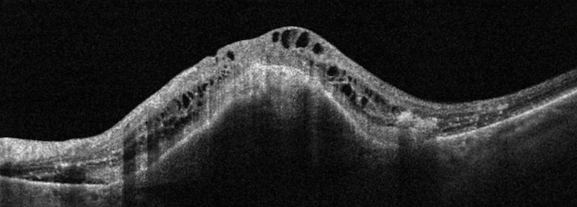 Macular scan. OCT B-scan — Impression: age-related macular degeneration.